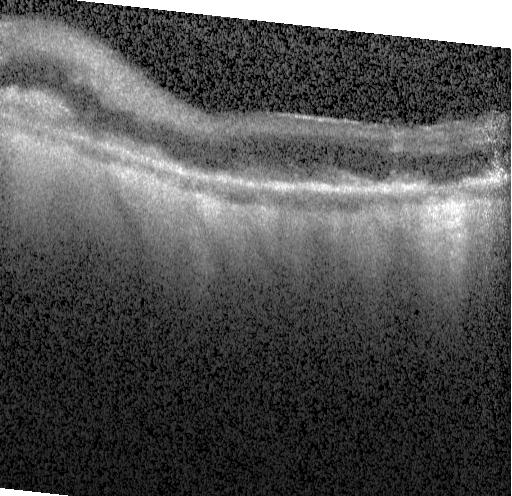
Horizontal scan through the fovea · OCT B-scan · spectral-domain OCT · acquired on a Heidelberg Spectralis.
Finding: CNV.